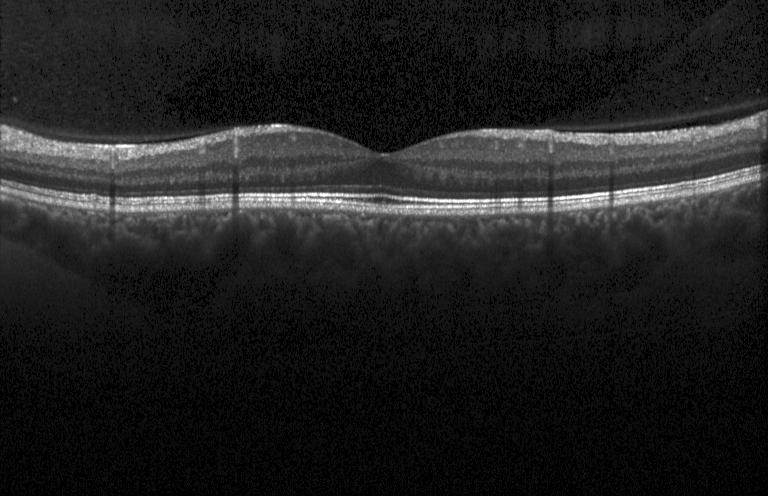
This B-scan demonstrates no evidence of CNV, DME, or drusen.